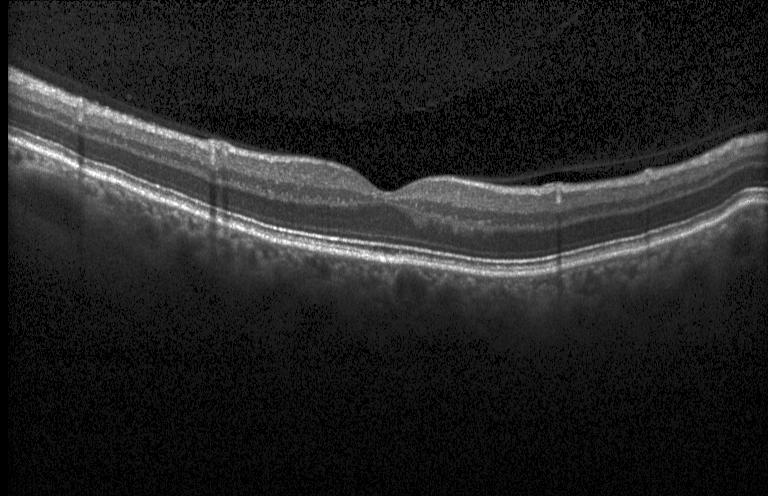 Retinal OCT cross-section. OCT finding: no choroidal neovascularization, diabetic macular edema, or drusen.